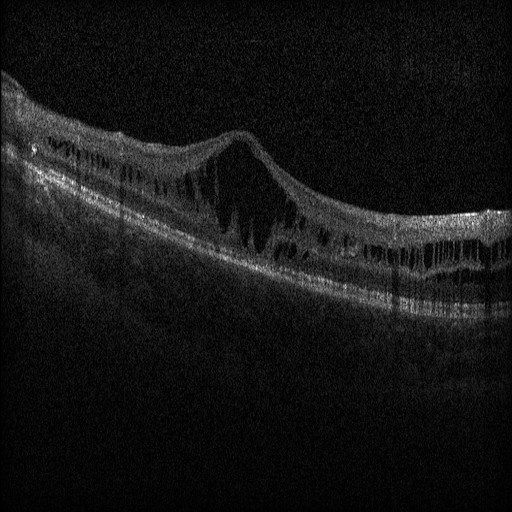
Horizontal scan through the fovea; Heidelberg Spectralis OCT system; retinal OCT cross-section.
Assessment: diabetic macular edema.